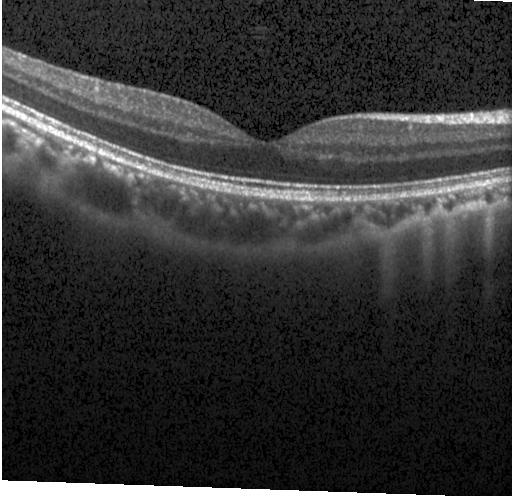

Retinal OCT cross-section showing no choroidal neovascularization, no diabetic macular edema, and no drusen.